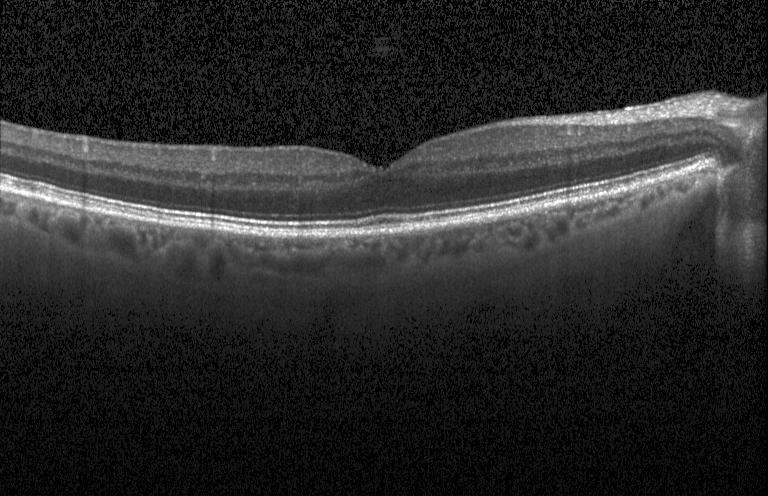

SD-OCT · instrument: Heidelberg Spectralis · OCT B-scan
OCT finding: neither choroidal neovascularization, diabetic macular edema, nor drusen.